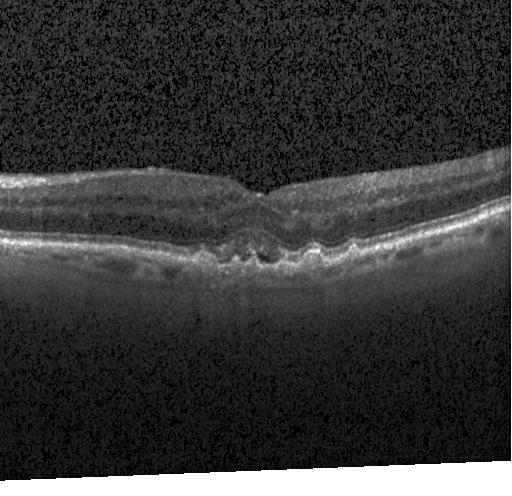 Spectral-domain OCT B-scan: choroidal neovascularization (CNV).